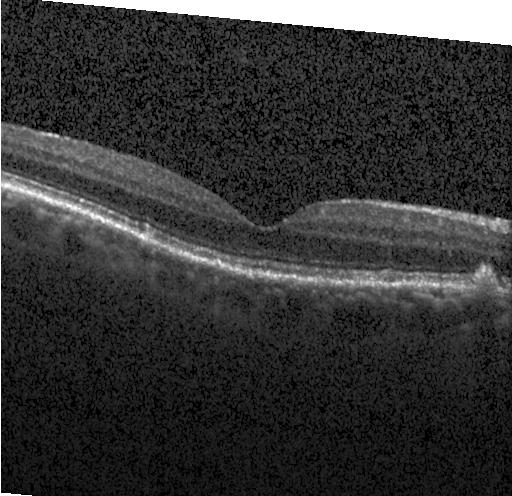 Macular OCT demonstrating sub-RPE drusenoid deposits.